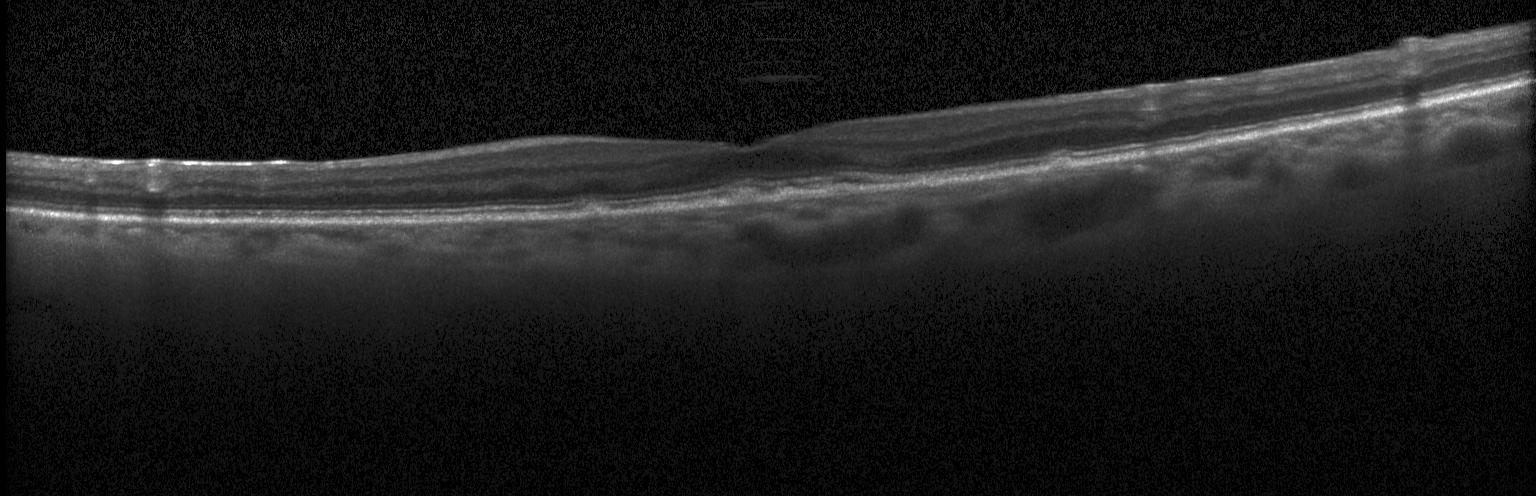
OCT scan showing drusen.